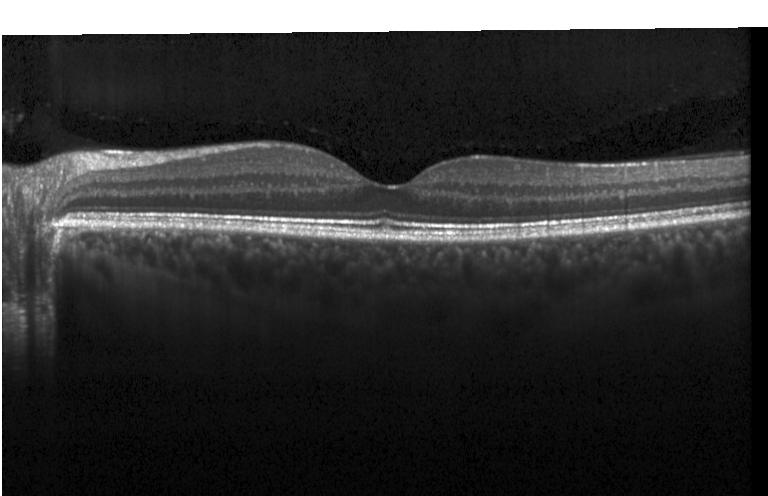 Through the macula; retinal OCT B-scan; Heidelberg Spectralis; SD-OCT
Impression: neither choroidal neovascularization, diabetic macular edema, nor drusen.